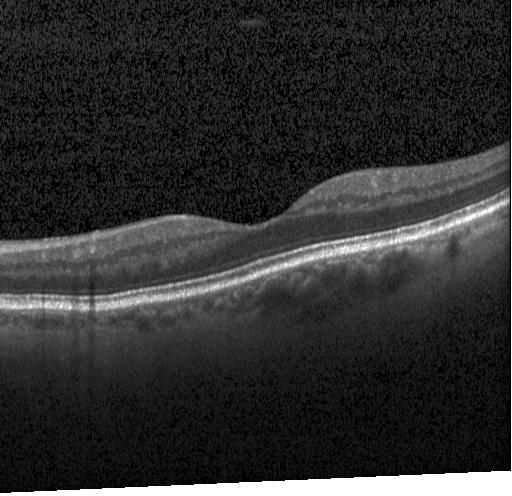
Instrument: Heidelberg Spectralis, optical coherence tomography scan, through the macula, SD-OCT — Neither CNV, DME, nor drusen.